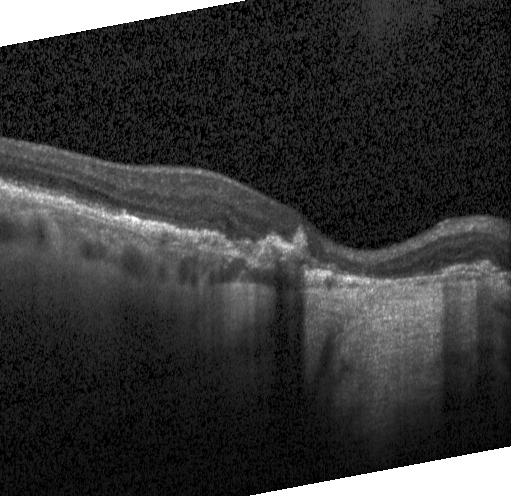

OCT line scan.
Impression: choroidal neovascularization (CNV).